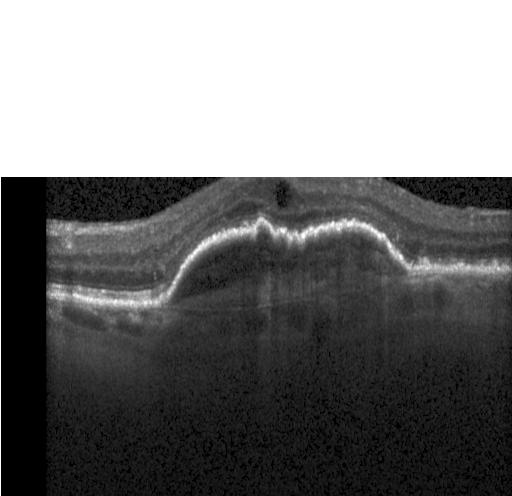 SD-OCT, retinal OCT cross-section, Heidelberg Spectralis.
Impression: CNV.